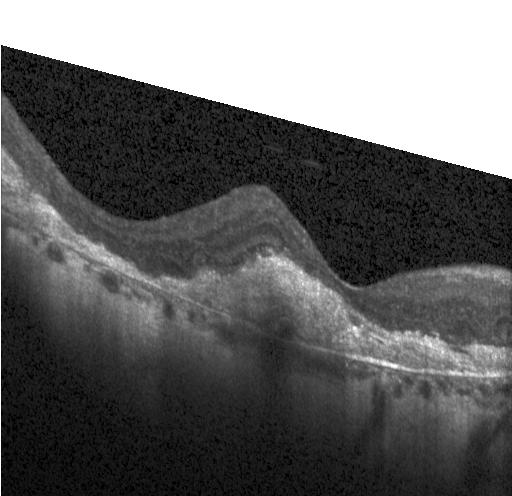

Macular OCT: a choroidal neovascular membrane.